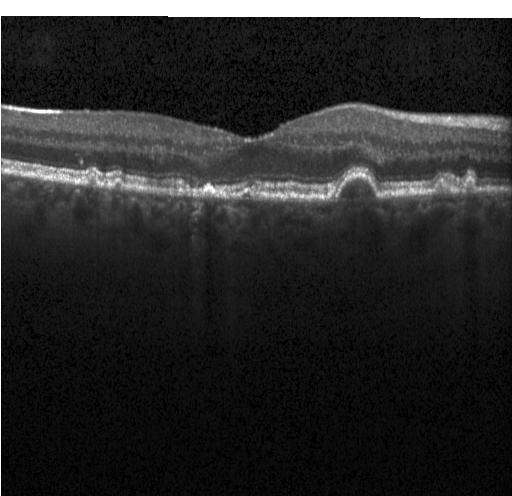
Acquired on a Heidelberg Spectralis · retinal OCT cross-section · spectral-domain optical coherence tomography · macular scan
The scan shows multiple drusen.